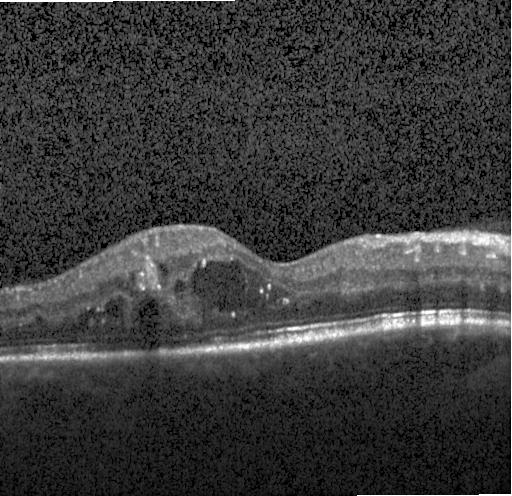

Macular OCT demonstrating diabetic macular edema (DME).